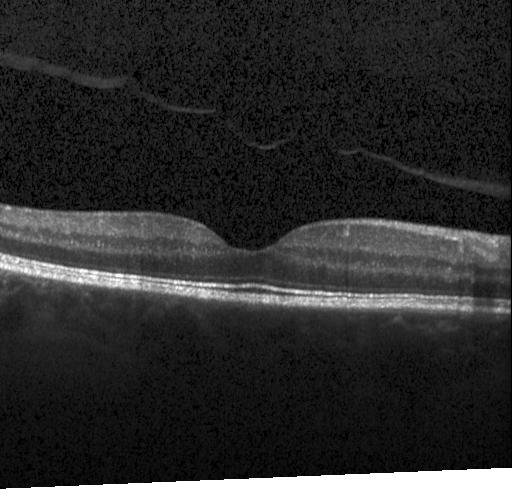 Dx: no evidence of choroidal neovascularization, diabetic macular edema, or drusen.